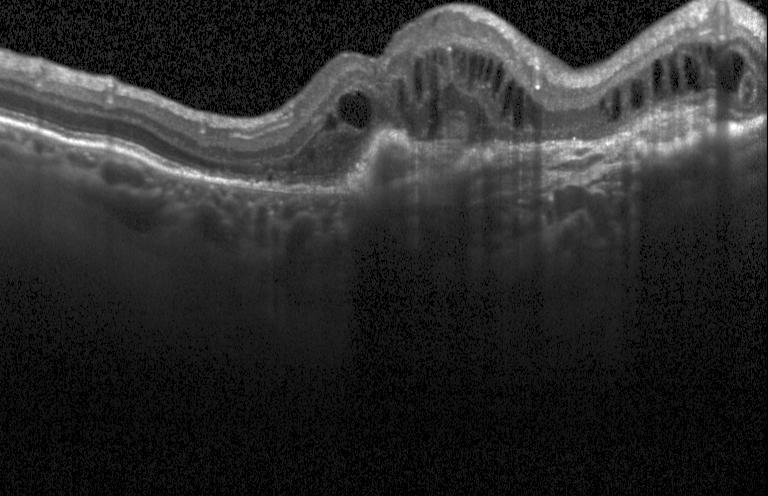

Spectral-domain OCT B-scan: choroidal neovascularization.